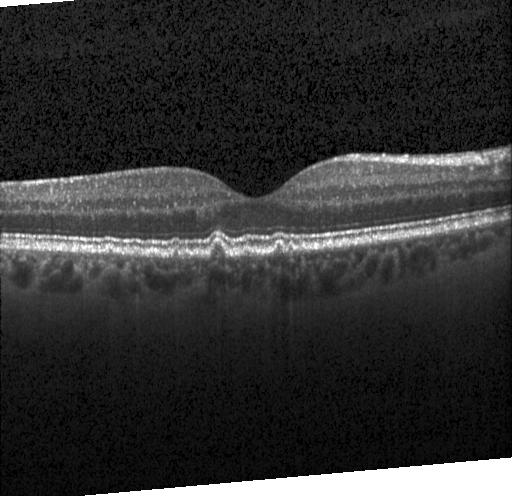

Diagnosis: sub-RPE drusenoid deposits.